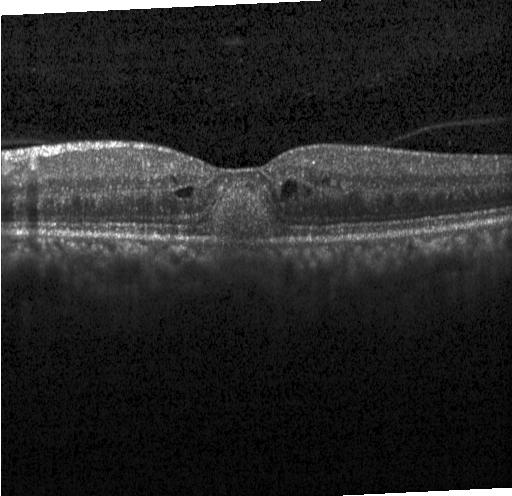 Finding: choroidal neovascularization (CNV).